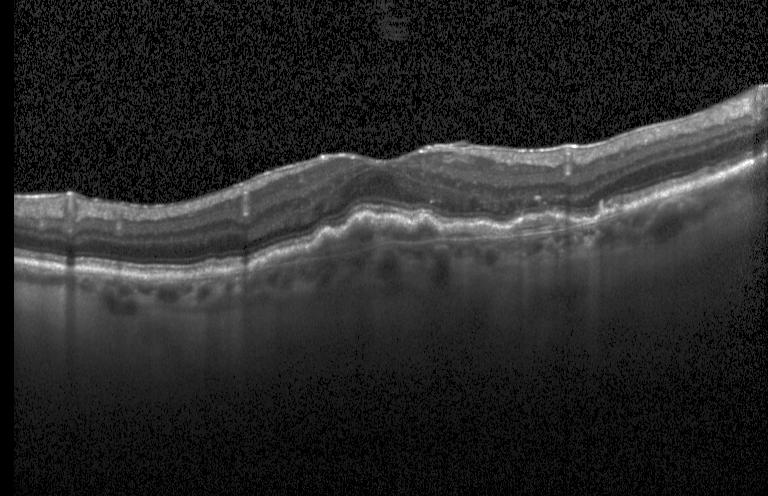
OCT B-scan. Spectral-domain OCT
Impression: a choroidal neovascular membrane.